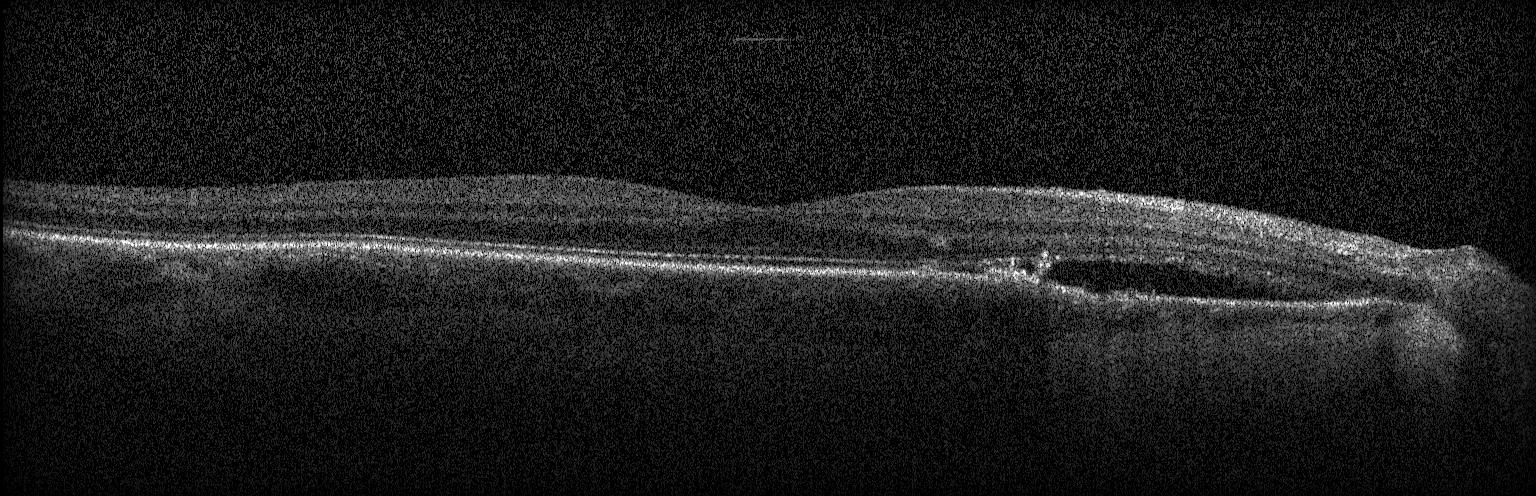

Macular scan; spectral-domain OCT; acquired on a Heidelberg Spectralis; optical coherence tomography B-scan
Diagnosis: choroidal neovascularization (CNV).